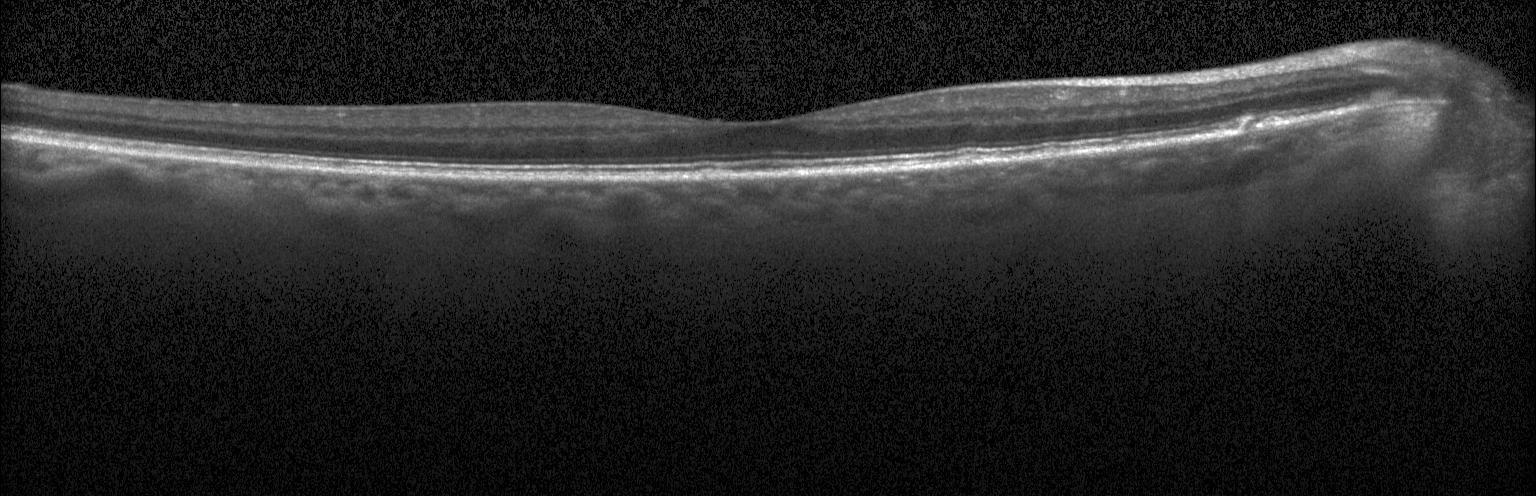

Macular OCT: neither choroidal neovascularization, diabetic macular edema, nor drusen.